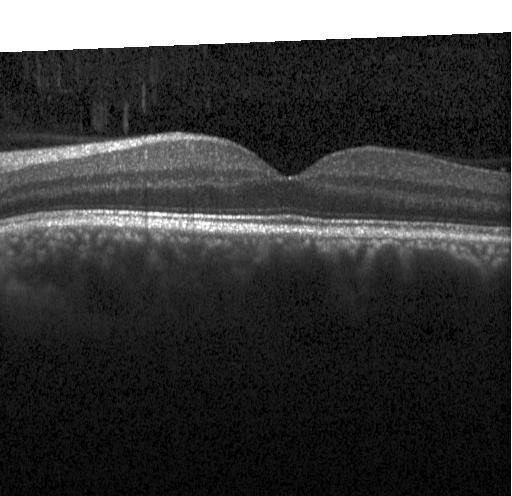

OCT line scan. Spectral-domain optical coherence tomography. Acquired on a Heidelberg Spectralis. Macular scan.
Finding: neither choroidal neovascularization, diabetic macular edema, nor drusen.